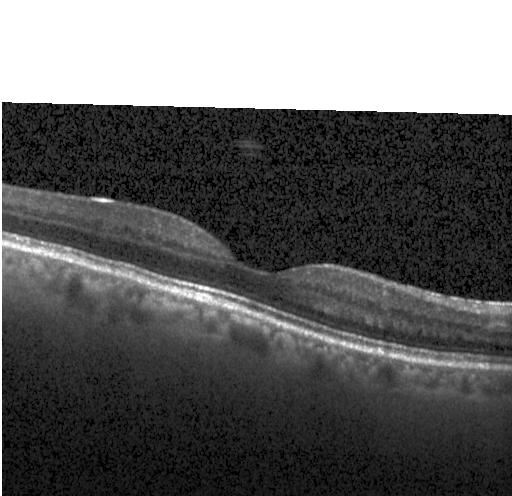 Spectral-domain optical coherence tomography · Heidelberg Spectralis OCT system · optical coherence tomography scan. Diagnosis: no evidence of CNV, DME, or drusen.